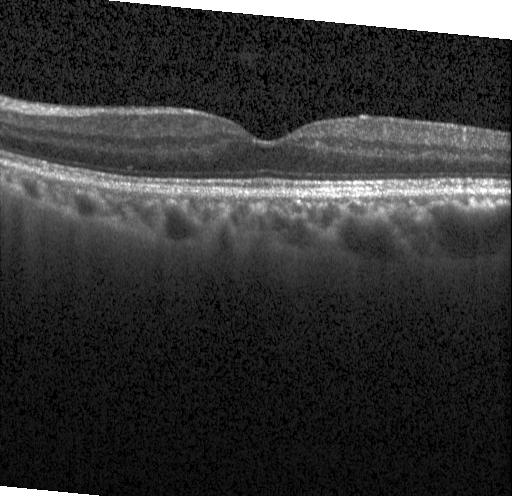 Impression: neither CNV, DME, nor drusen.